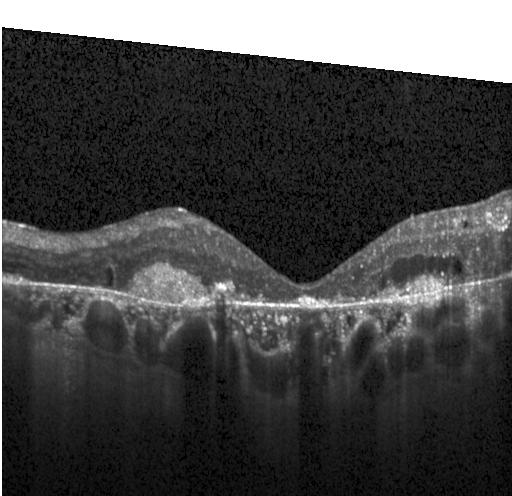 Diagnosis: choroidal neovascularization.